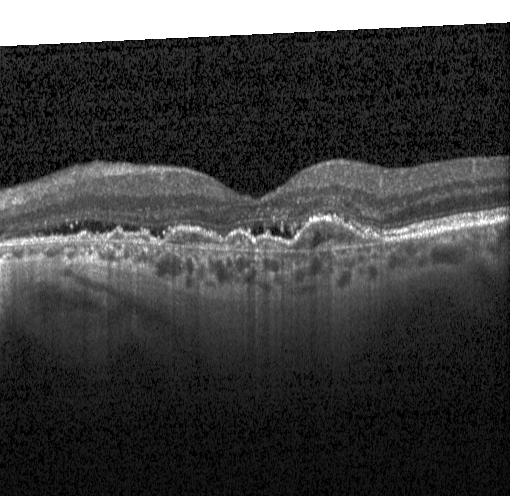 Impression: CNV.